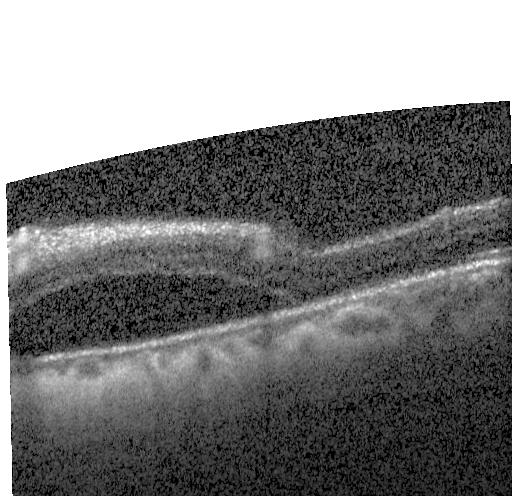
Optical coherence tomography scan · through the macula — Macular OCT: choroidal neovascularization.